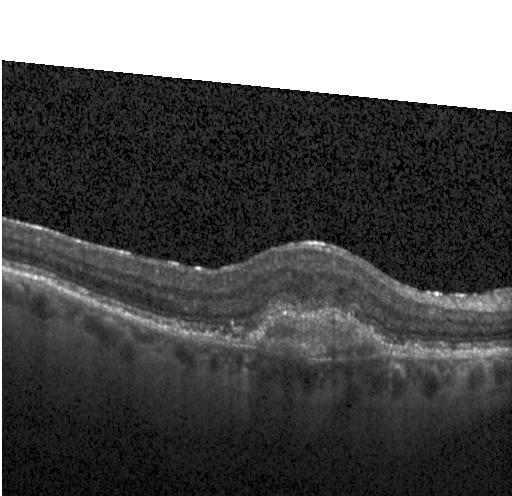

Spectral-domain optical coherence tomography · Heidelberg Spectralis · retinal OCT cross-section
Finding: choroidal neovascularization.